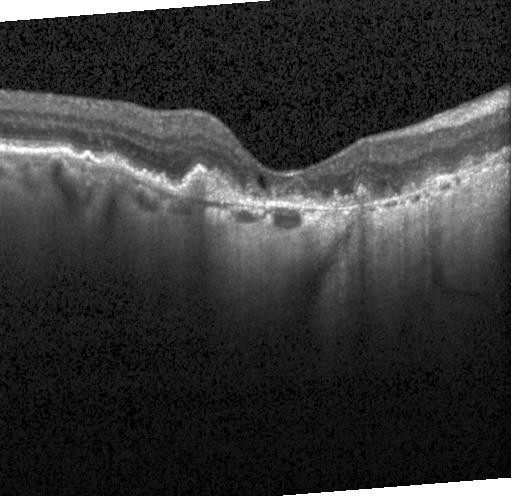 Dx: a choroidal neovascular membrane.